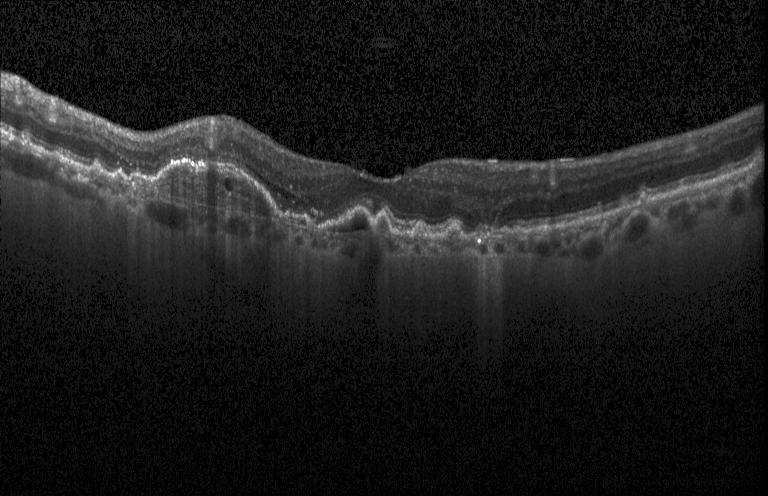

Optical coherence tomography scan; Heidelberg Spectralis OCT system; fovea-centered; spectral-domain OCT. Impression: CNV.